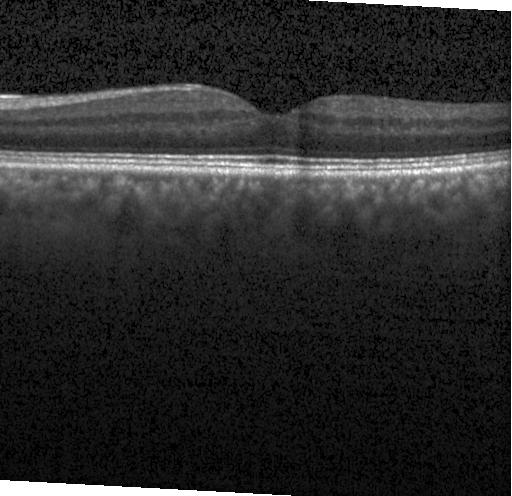
OCT finding: no choroidal neovascularization, no diabetic macular edema, and no drusen.